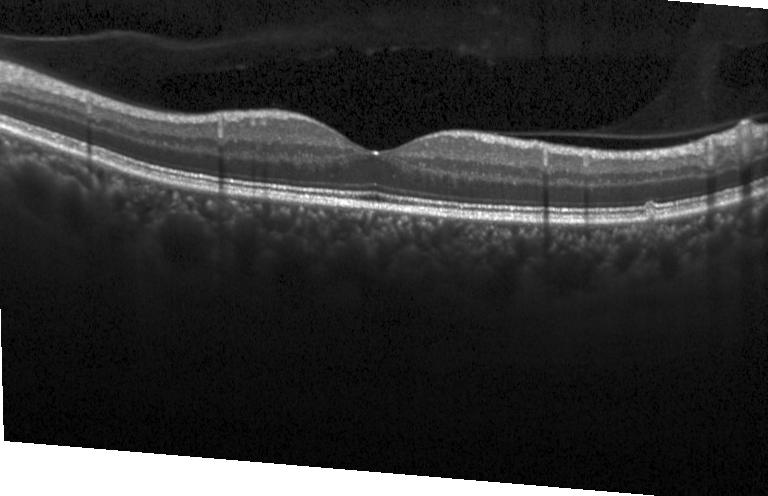 Optical coherence tomography B-scan · macular scan
Impression: neither choroidal neovascularization, diabetic macular edema, nor drusen.